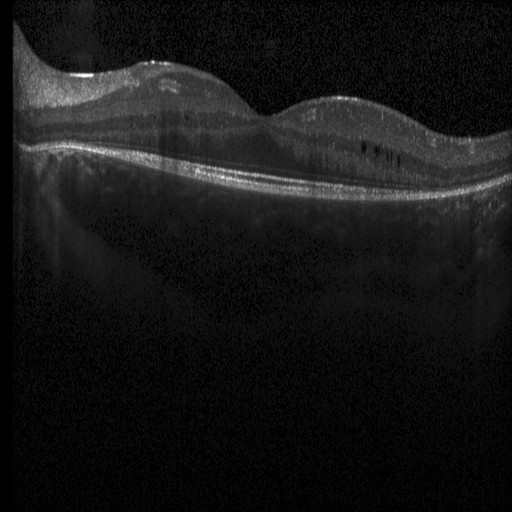
Heidelberg Spectralis OCT system; spectral-domain optical coherence tomography; OCT line scan.
Impression: diabetic macular edema.